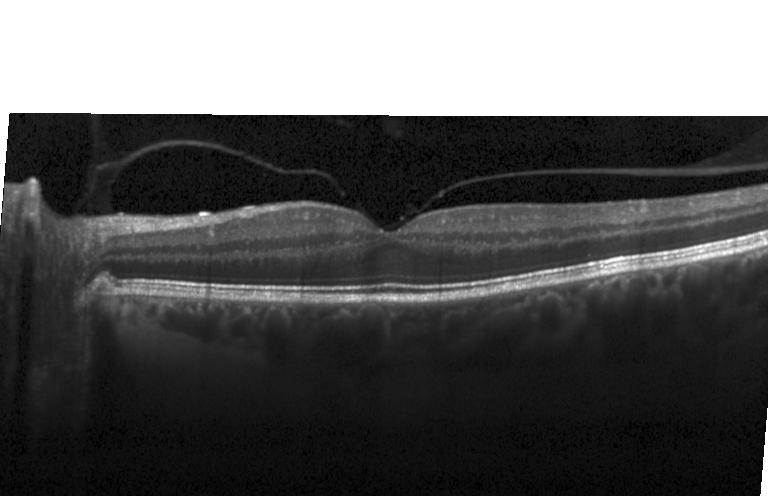 Retinal OCT B-scan. Impression: no choroidal neovascularization, diabetic macular edema, or drusen.